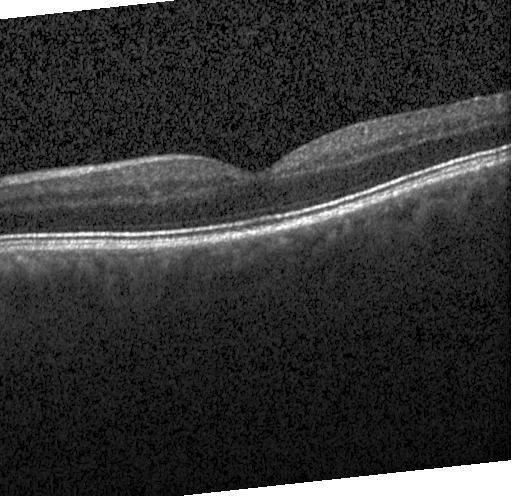
Finding: no choroidal neovascularization, diabetic macular edema, or drusen.